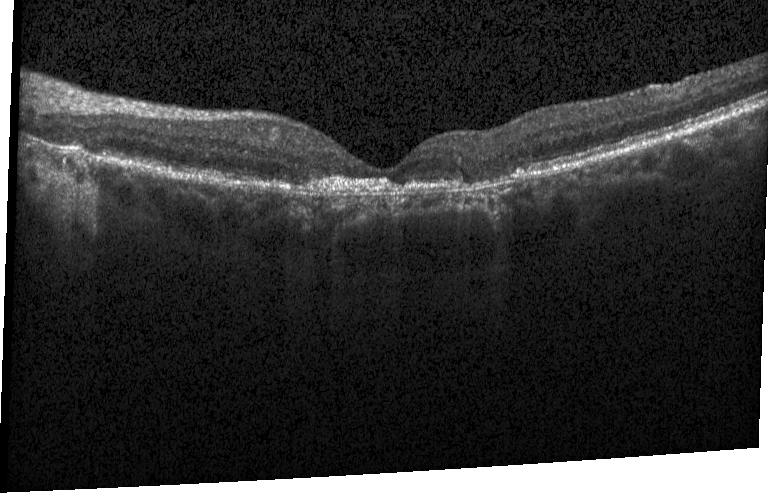 Optical coherence tomography B-scan. Horizontal scan through the fovea
Macular OCT: choroidal neovascularization (CNV).